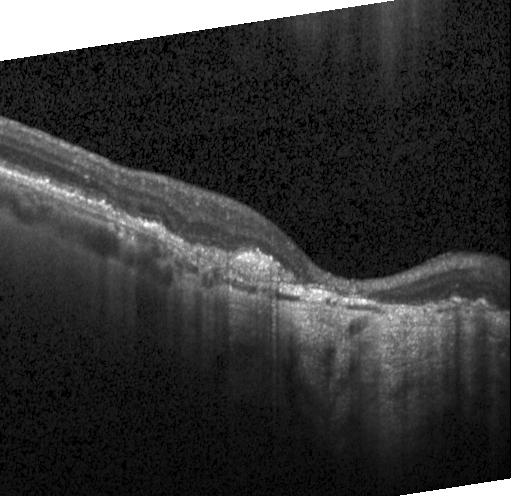

Impression: a choroidal neovascular membrane.